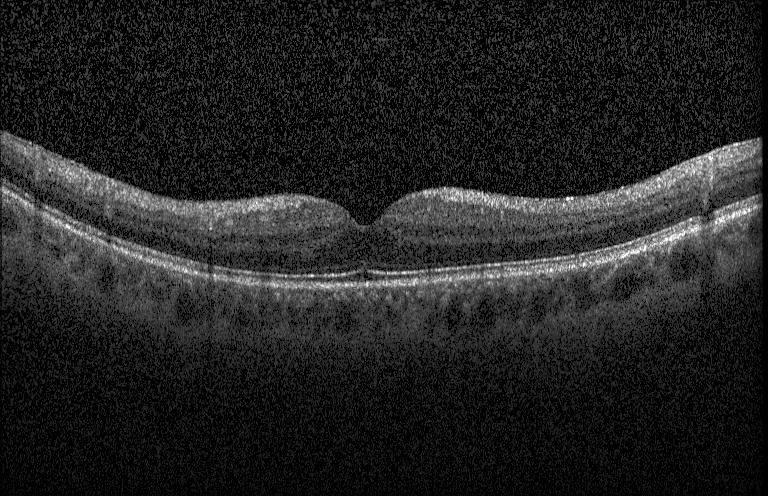

Instrument: Heidelberg Spectralis, OCT line scan, SD-OCT, macular scan. Finding: no CNV, DME, or drusen.